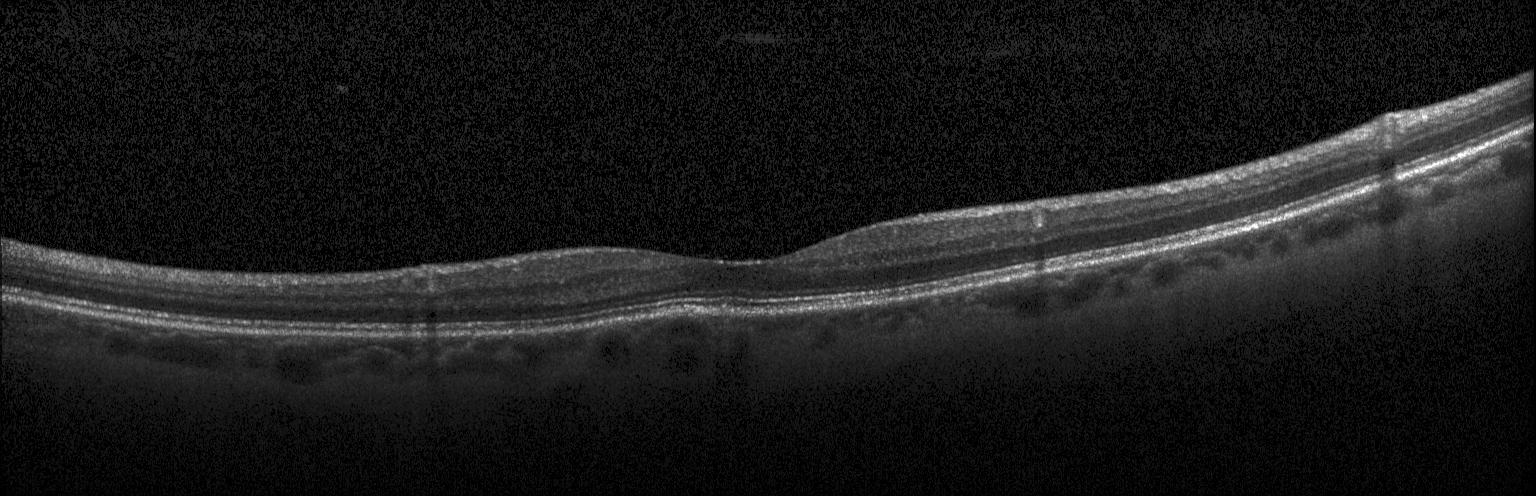
SD-OCT, retinal OCT B-scan, horizontal scan through the fovea. This B-scan demonstrates no choroidal neovascularization, no diabetic macular edema, and no drusen.